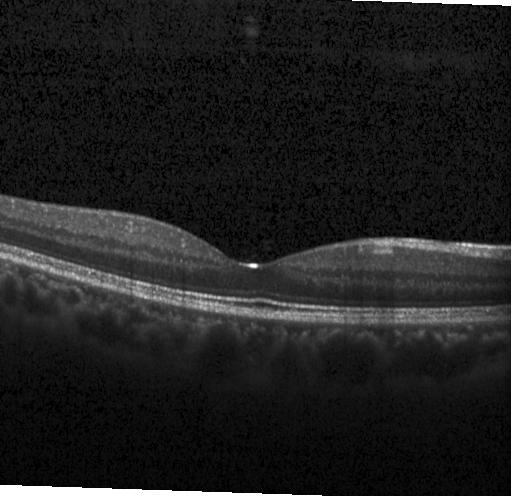 Acquired on a Heidelberg Spectralis; spectral-domain optical coherence tomography; optical coherence tomography scan; centered on the fovea. Dx: no choroidal neovascularization, no diabetic macular edema, and no drusen.